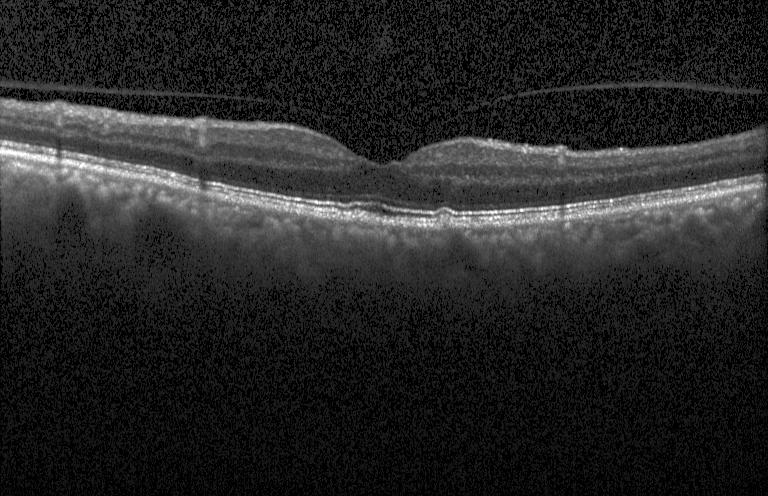
Optical coherence tomography B-scan
The scan shows multiple drusen.